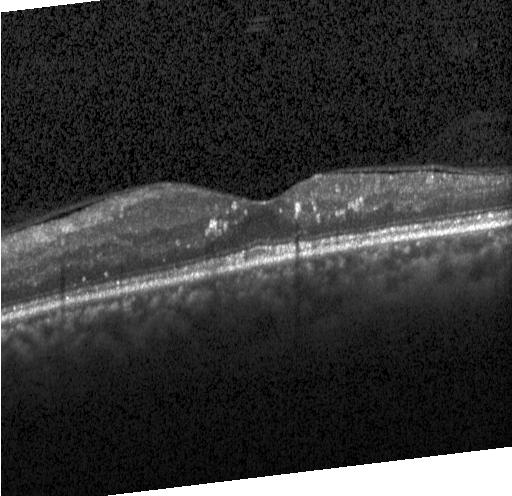 Finding: diabetic macular edema.